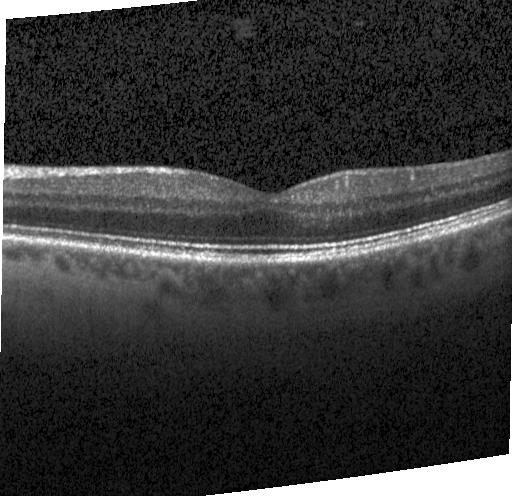

Heidelberg Spectralis. OCT B-scan. SD-OCT. Through the macula
Macular OCT: no CNV, DME, or drusen.